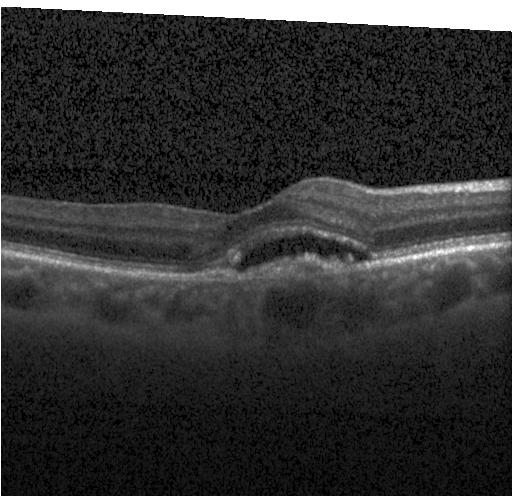

Retinal OCT cross-section, centered on the fovea, Heidelberg Spectralis OCT system, SD-OCT. Dx: CNV.